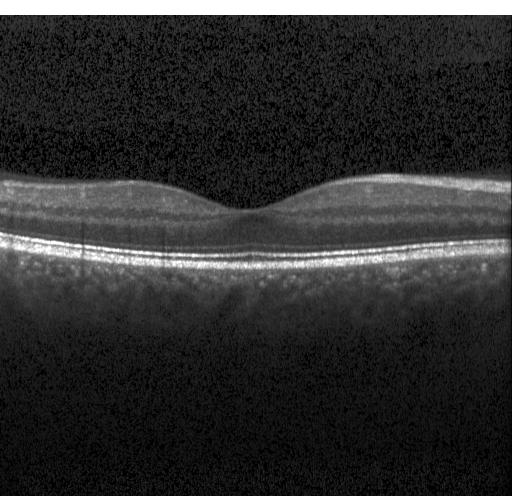 Retinal OCT B-scan, instrument: Heidelberg Spectralis, macular scan.
OCT finding: no choroidal neovascularization, diabetic macular edema, or drusen.